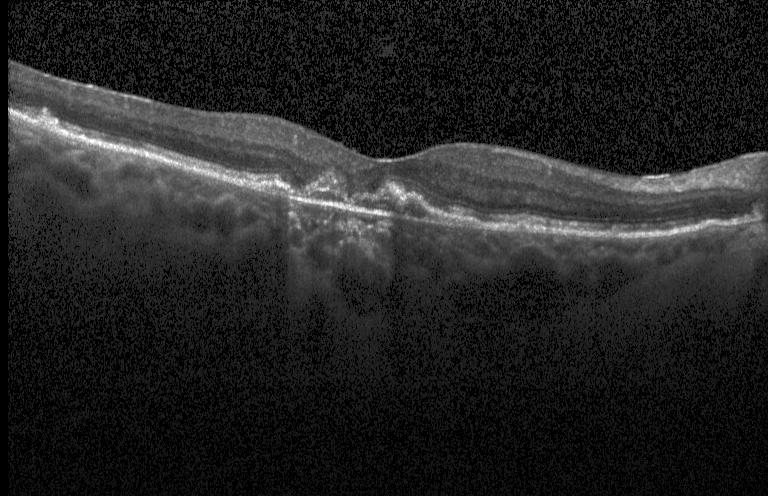 Diagnosis: CNV.